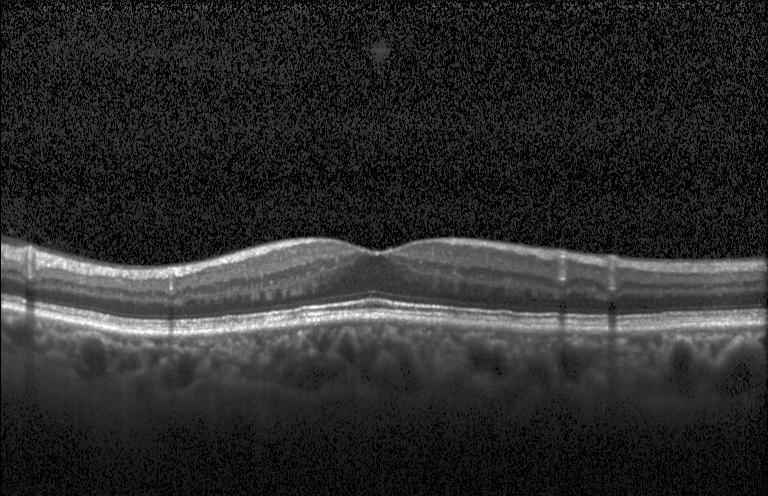
Retinal OCT cross-section · Heidelberg Spectralis OCT system · spectral-domain OCT · through the macula
This B-scan demonstrates no choroidal neovascularization, no diabetic macular edema, and no drusen.